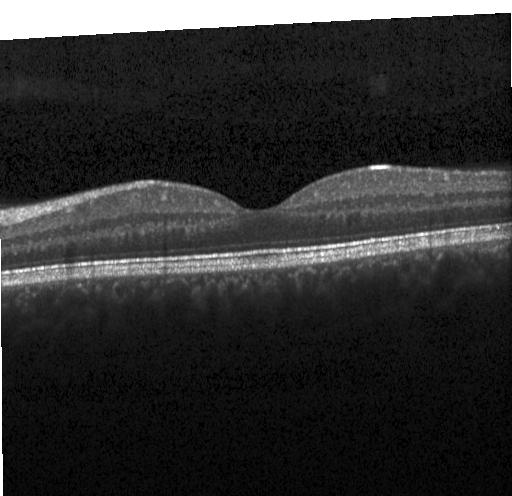
Retinal OCT B-scan.
The scan shows no evidence of CNV, DME, or drusen.